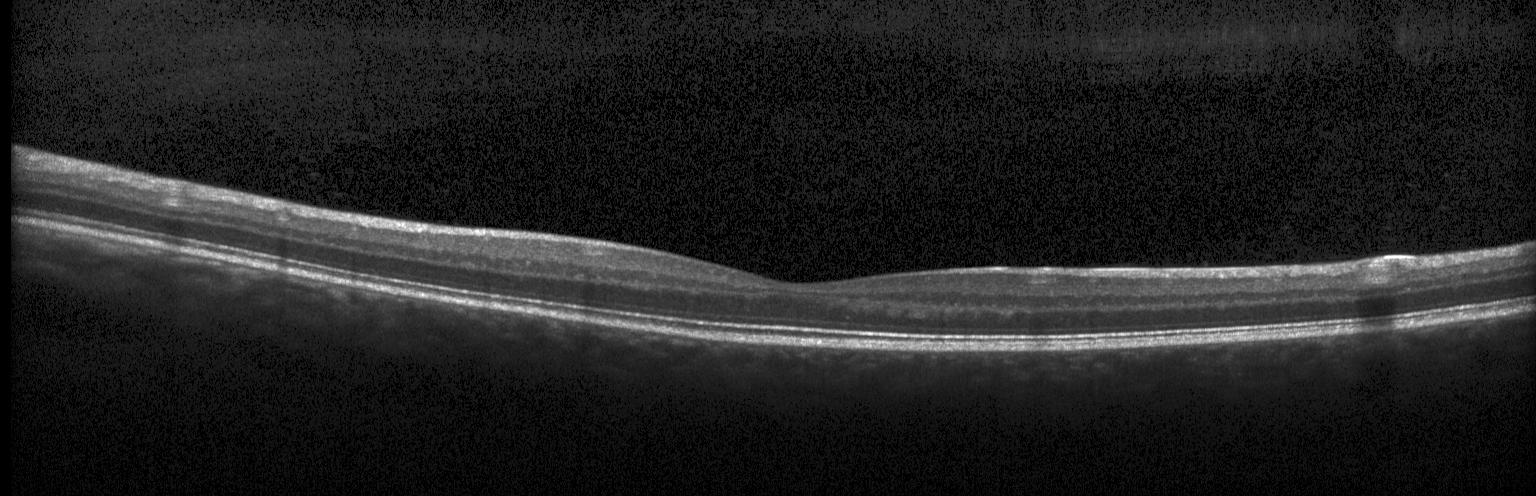 Optical coherence tomography B-scan. Centered on the fovea
Impression: neither choroidal neovascularization, diabetic macular edema, nor drusen.